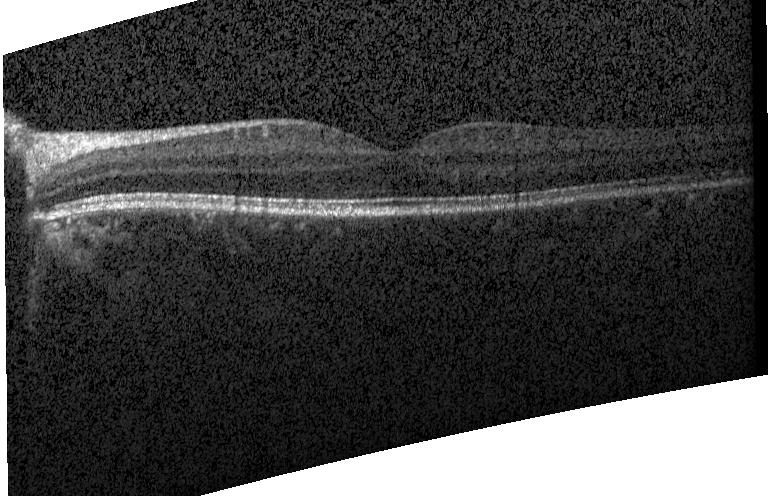

Finding: no CNV, no DME, and no drusen.